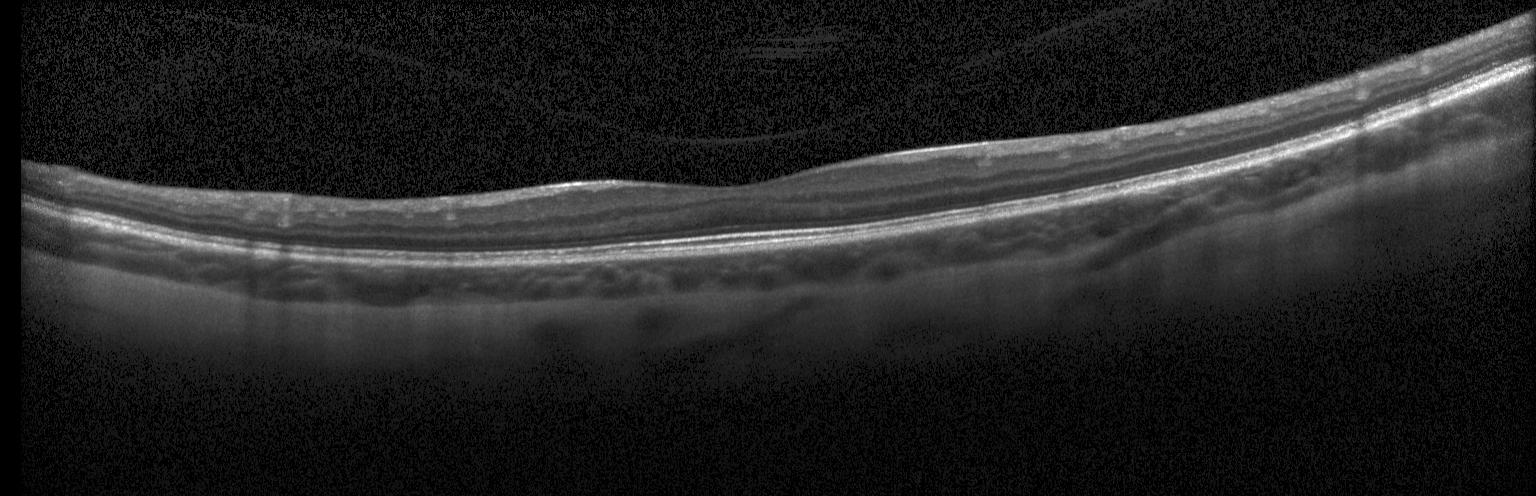

SD-OCT; horizontal scan through the fovea; OCT B-scan.
Assessment: no CNV, DME, or drusen.